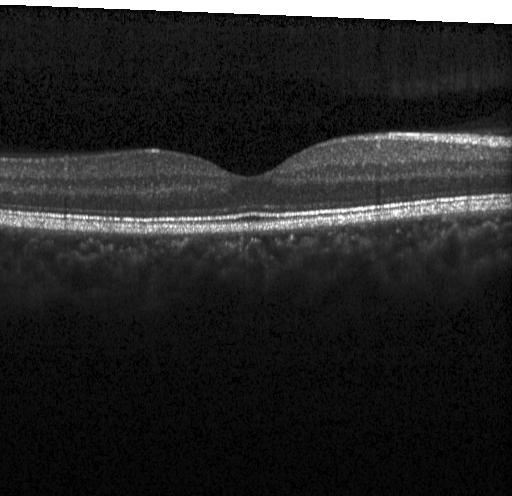
Macular OCT: no evidence of CNV, DME, or drusen.